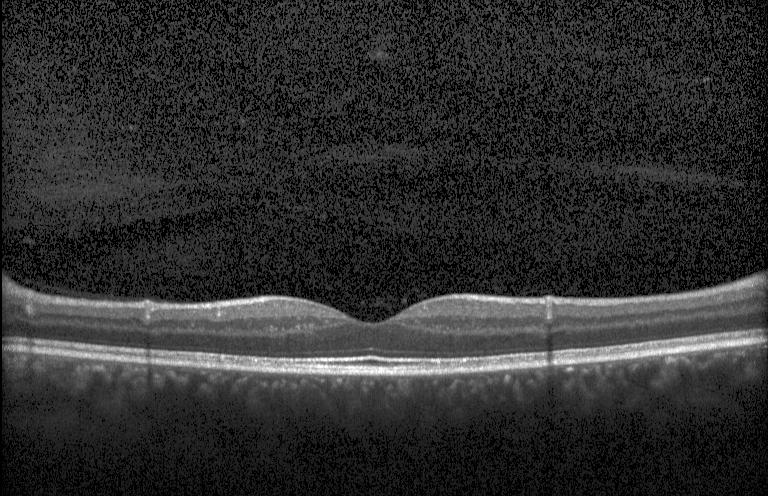

Impression: no choroidal neovascularization, diabetic macular edema, or drusen.